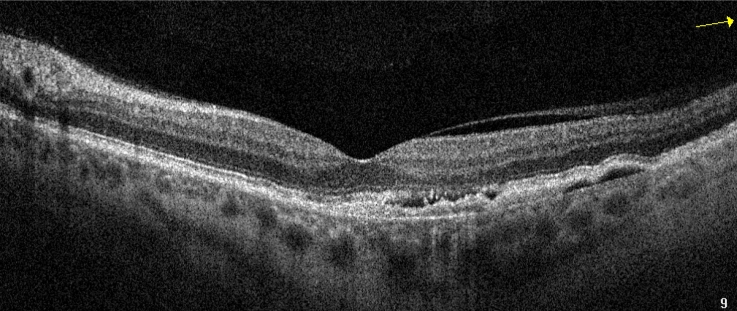

OCT B-scan; fovea-centered.
This B-scan demonstrates age-related macular degeneration.